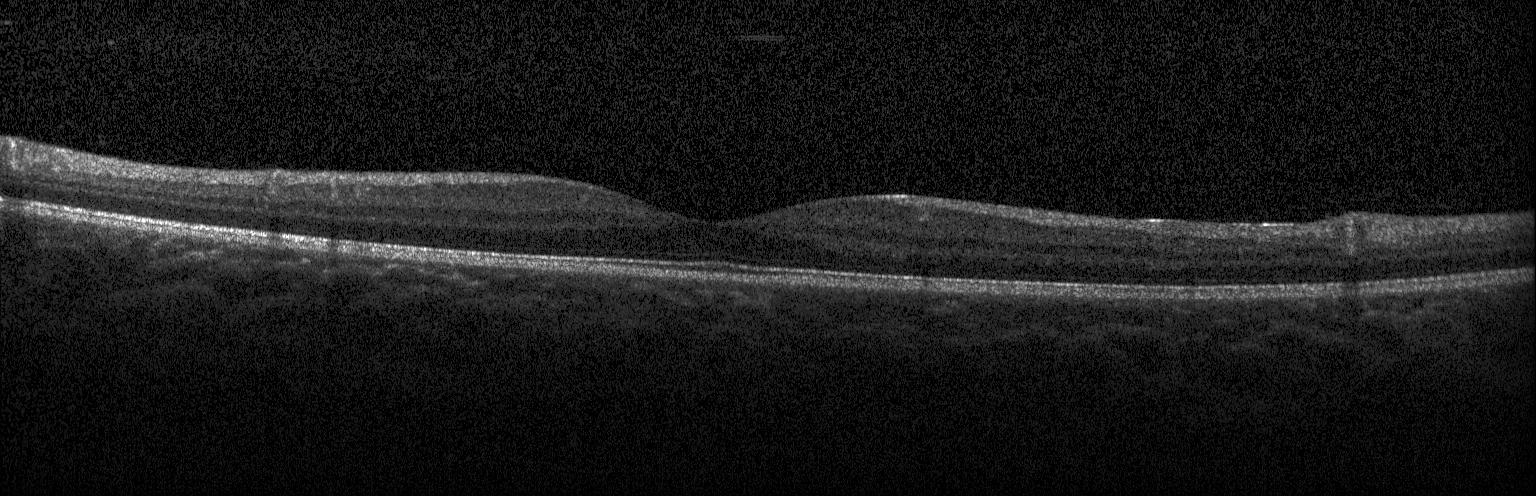

Impression: neither CNV, DME, nor drusen.